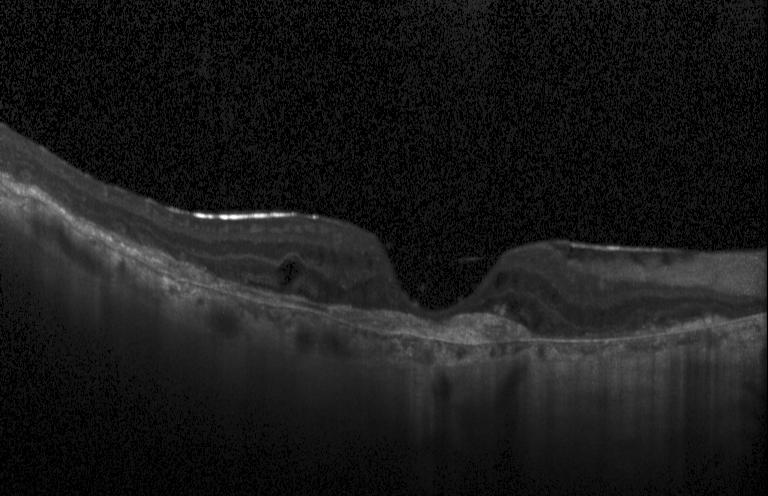

SD-OCT. Optical coherence tomography B-scan. Horizontal scan through the fovea. Impression: a choroidal neovascular membrane.